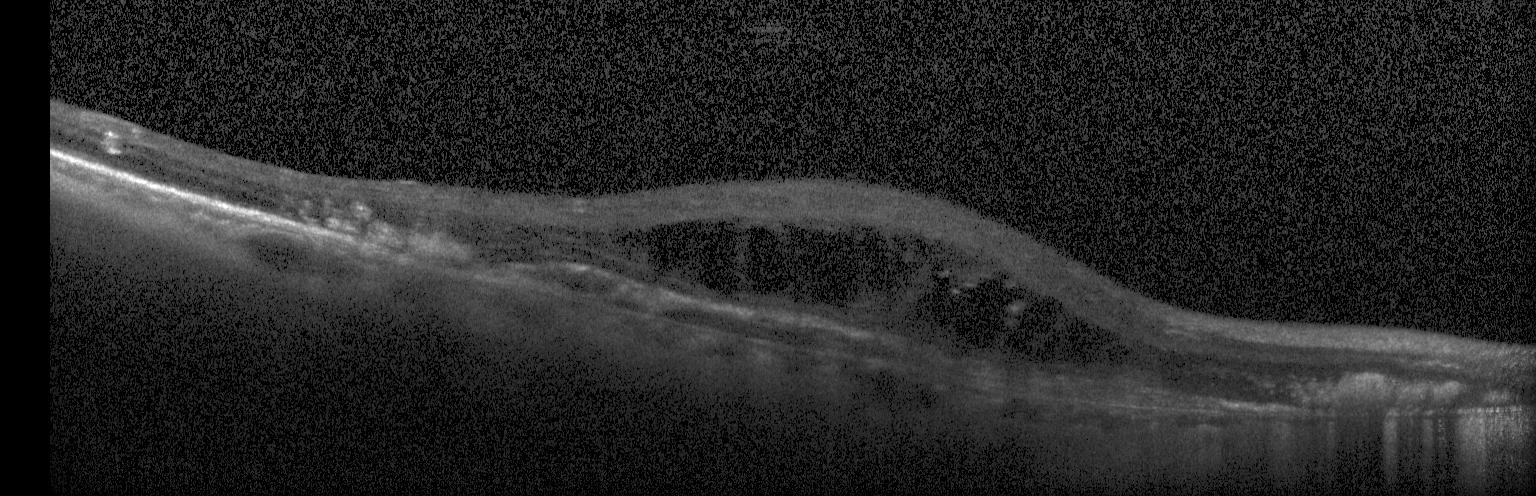 Spectral-domain OCT B-scan: choroidal neovascularization (CNV).